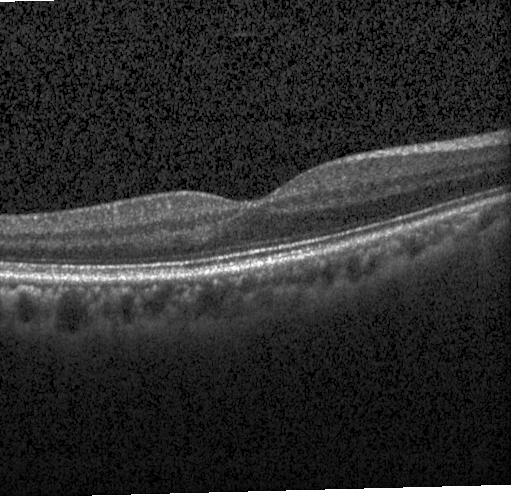

Retinal OCT B-scan, spectral-domain OCT, Heidelberg Spectralis OCT system. OCT finding: neither choroidal neovascularization, diabetic macular edema, nor drusen.